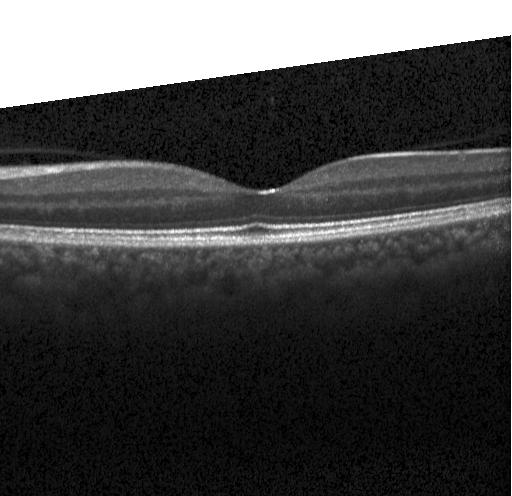
Retinal OCT B-scan
No choroidal neovascularization, no diabetic macular edema, and no drusen.